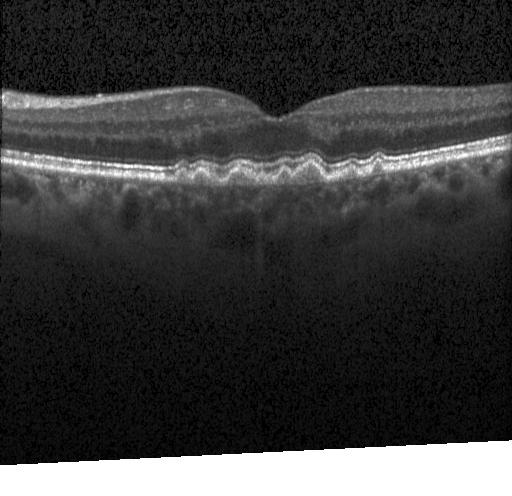 Retinal OCT cross-section; Heidelberg Spectralis OCT system.
Diagnosis: multiple drusen.